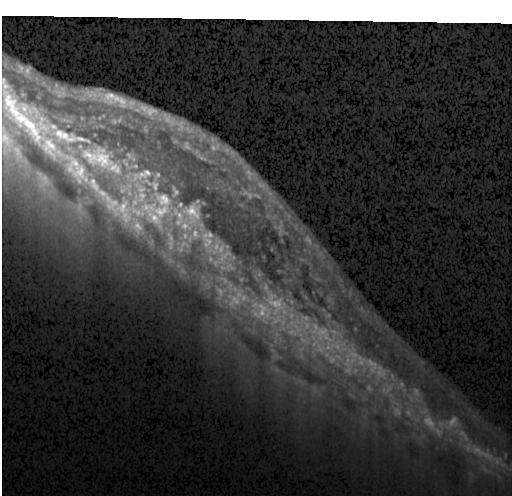
OCT finding: a choroidal neovascular membrane.